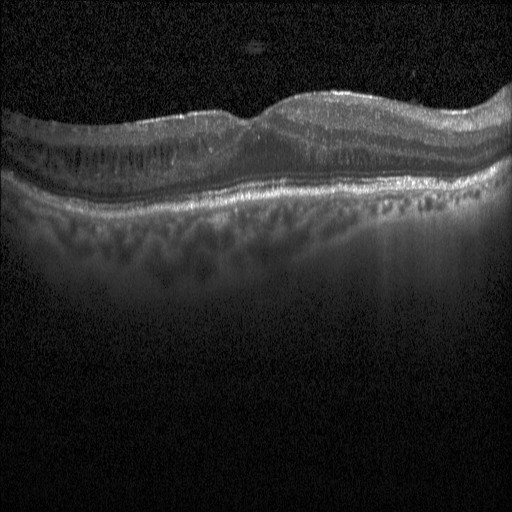 OCT finding: diabetic macular edema.